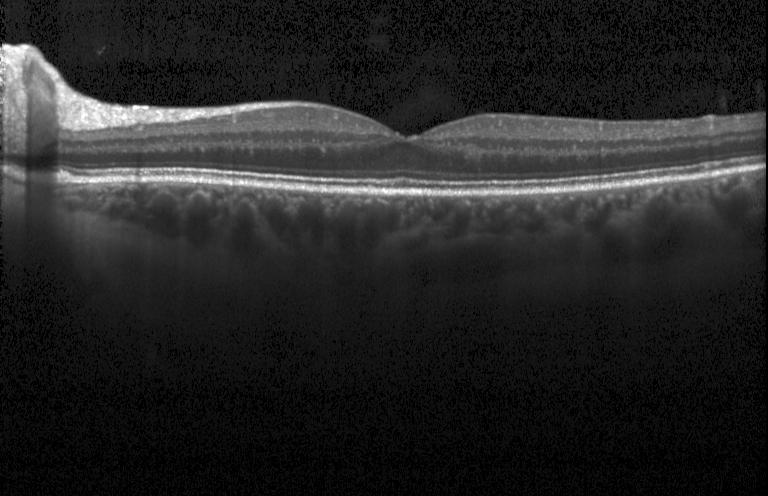
Spectral-domain OCT B-scan: no choroidal neovascularization, diabetic macular edema, or drusen.